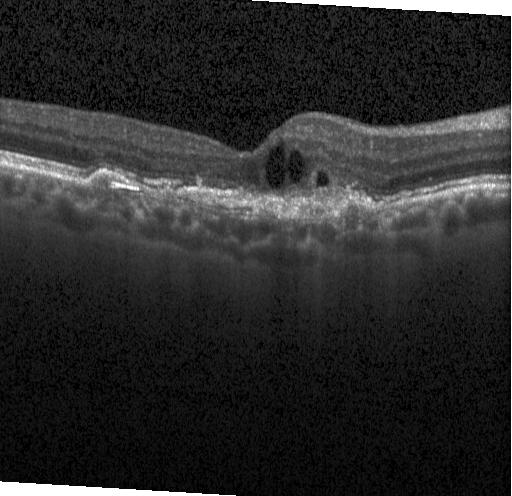 OCT B-scan showing a choroidal neovascular membrane.